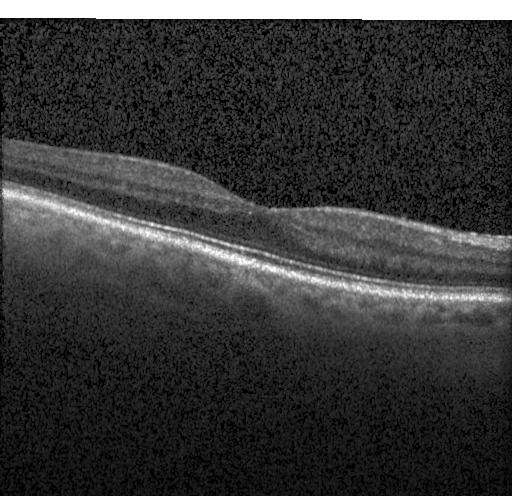

OCT finding: no choroidal neovascularization, no diabetic macular edema, and no drusen.